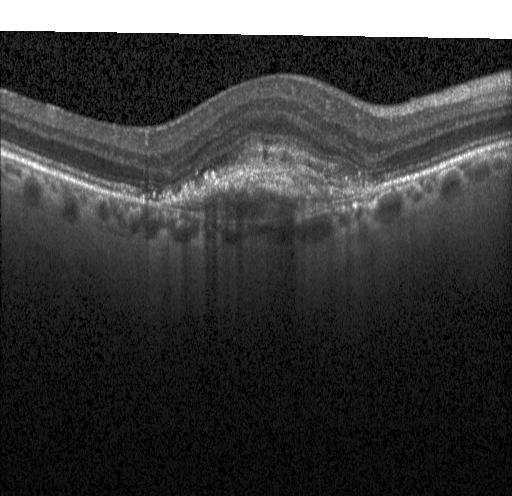
Impression: choroidal neovascularization.